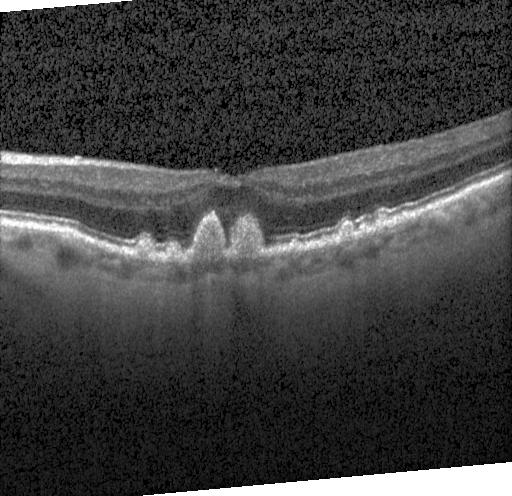
This B-scan demonstrates multiple drusen.